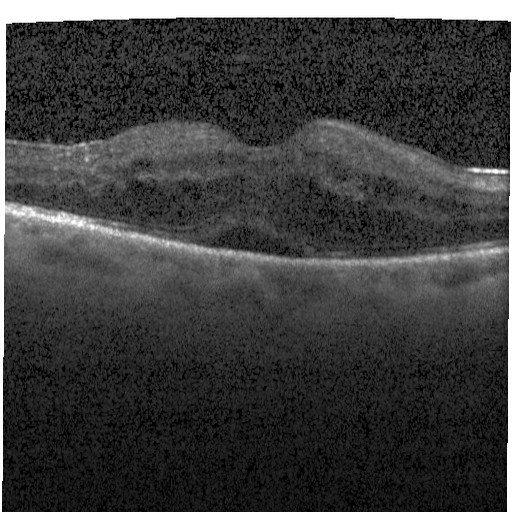

OCT B-scan · spectral-domain OCT · macular scan
Diagnosis: diabetic macular edema.